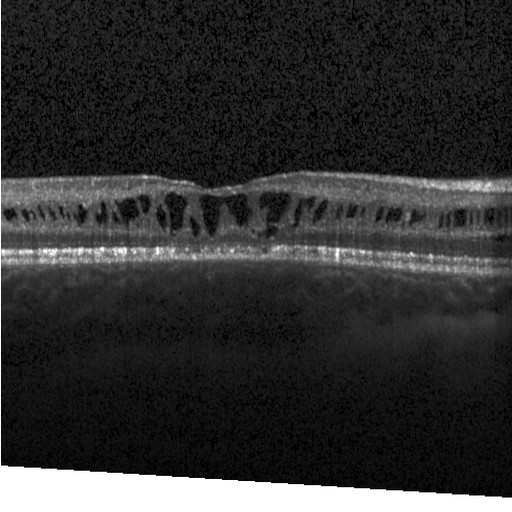

Optical coherence tomography B-scan — This B-scan demonstrates diabetic macular edema (DME).